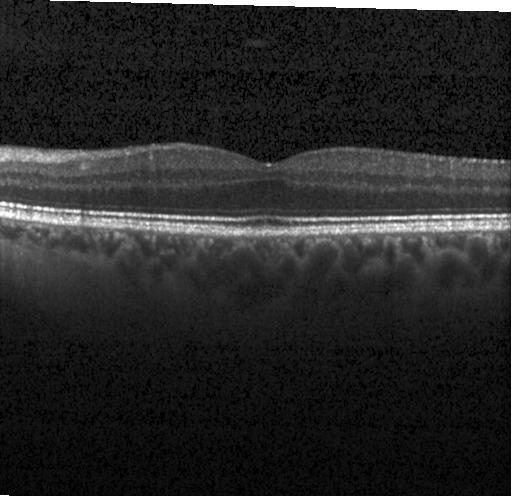 Instrument: Heidelberg Spectralis; OCT line scan; spectral-domain OCT; horizontal scan through the fovea.
OCT finding: neither choroidal neovascularization, diabetic macular edema, nor drusen.